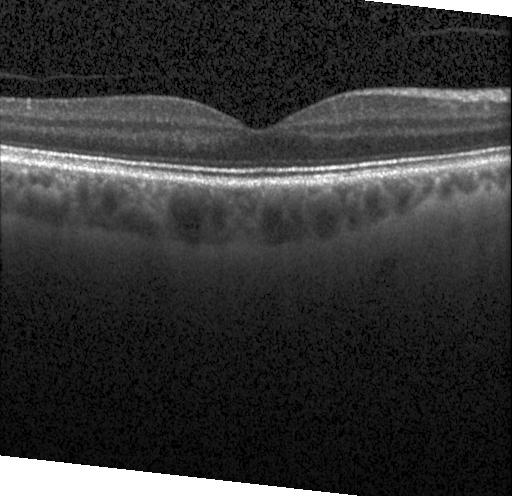 Optical coherence tomography scan
Finding: no choroidal neovascularization, no diabetic macular edema, and no drusen.